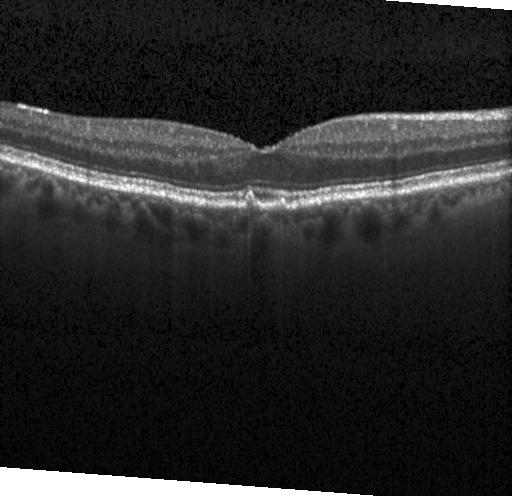
Impression: drusen.